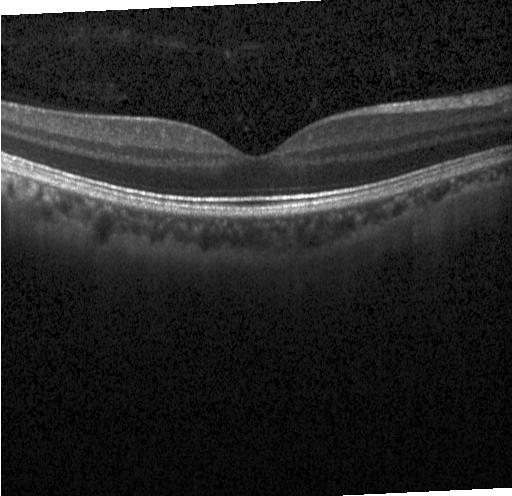
The scan shows no CNV, DME, or drusen.